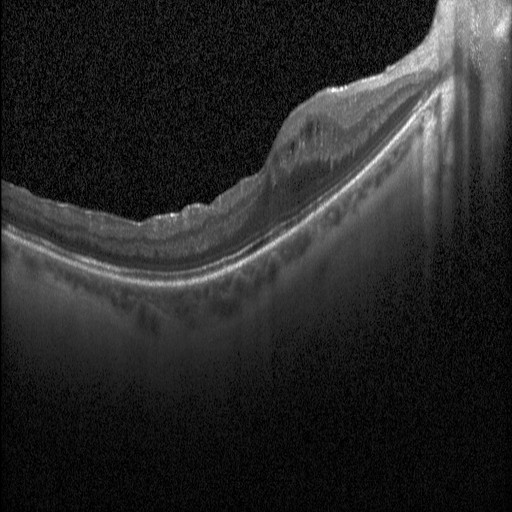 Macular OCT: diabetic macular edema.